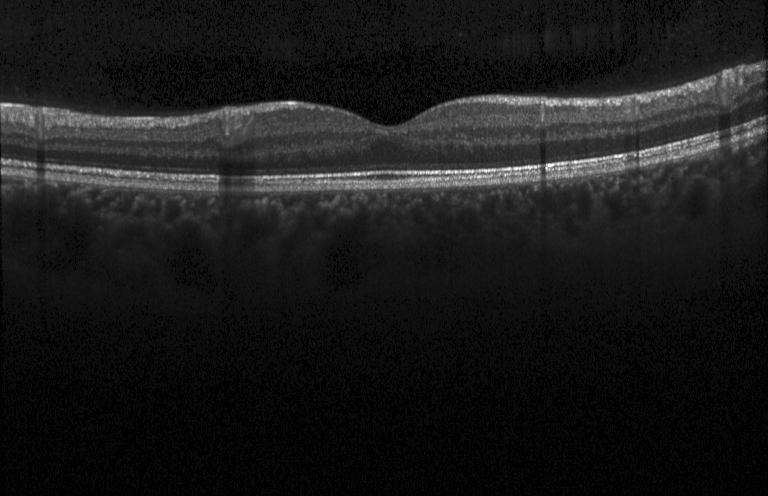

OCT B-scan showing neither choroidal neovascularization, diabetic macular edema, nor drusen.